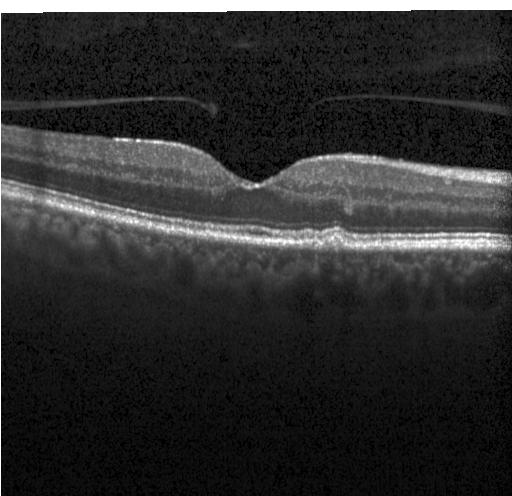 Horizontal scan through the fovea. Acquired on a Heidelberg Spectralis. Spectral-domain OCT. OCT B-scan
Diagnosis: sub-RPE drusenoid deposits.